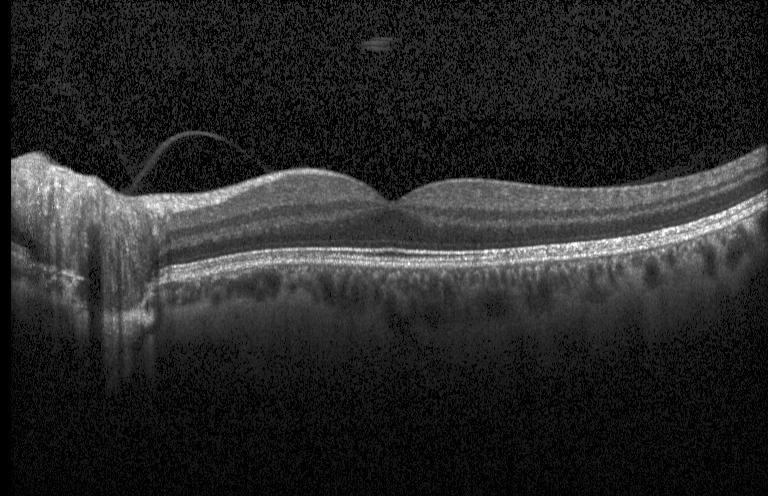

Retinal OCT cross-section showing no choroidal neovascularization, diabetic macular edema, or drusen.